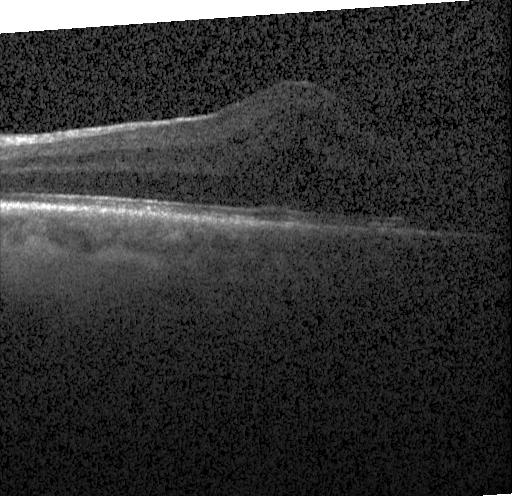

SD-OCT, OCT line scan, fovea-centered. OCT finding: DME.